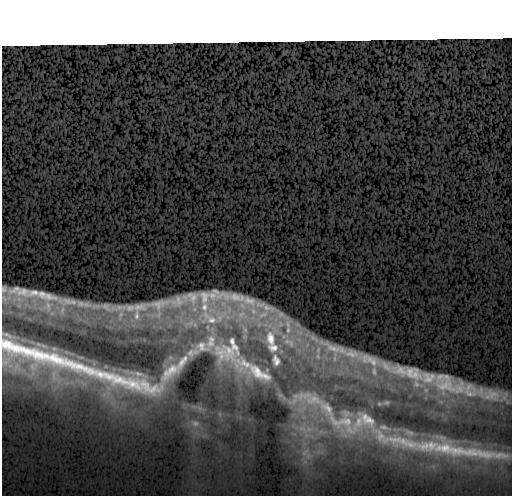

Retinal OCT cross-section showing choroidal neovascularization (CNV).